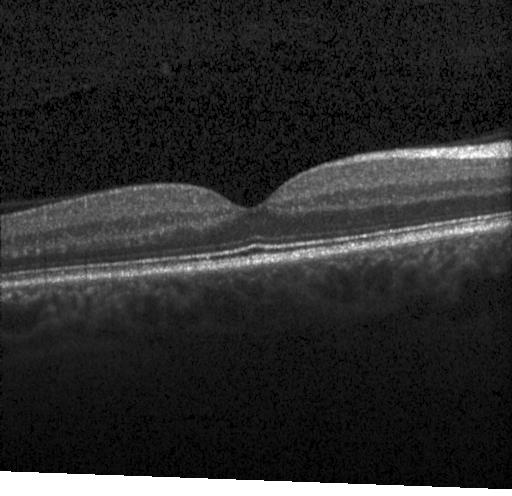
Impression: no choroidal neovascularization, diabetic macular edema, or drusen.